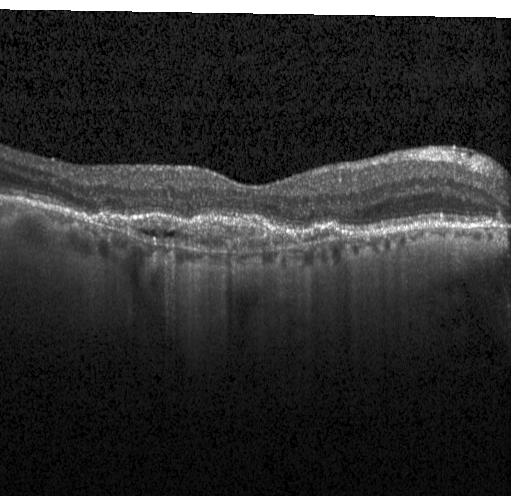 Diagnosis: choroidal neovascularization.